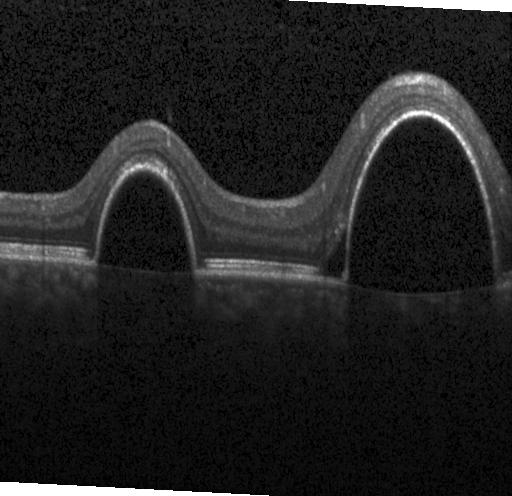

Optical coherence tomography B-scan, centered on the fovea — Impression: choroidal neovascularization.